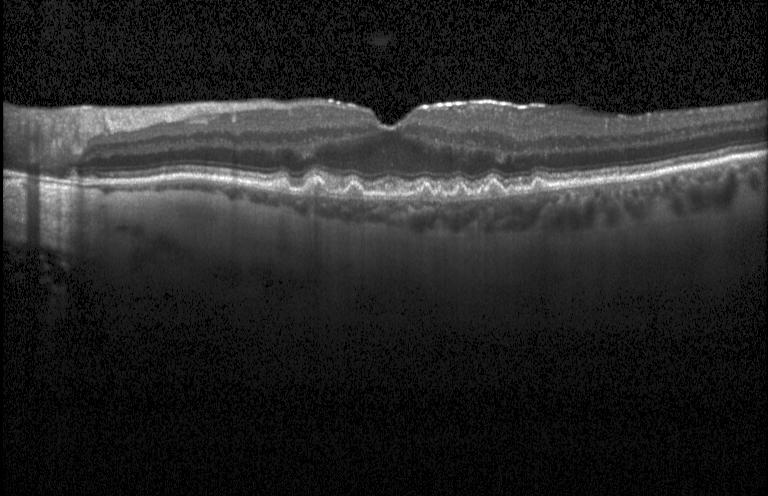

OCT finding: sub-RPE drusenoid deposits.